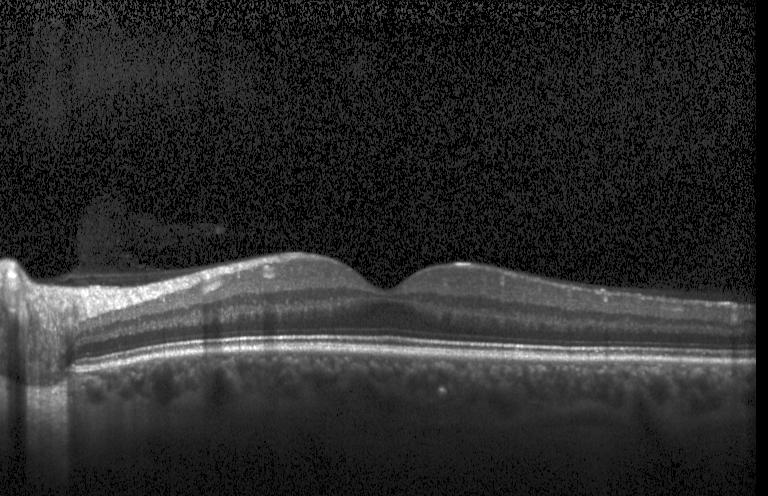

Macular OCT: no choroidal neovascularization, no diabetic macular edema, and no drusen.